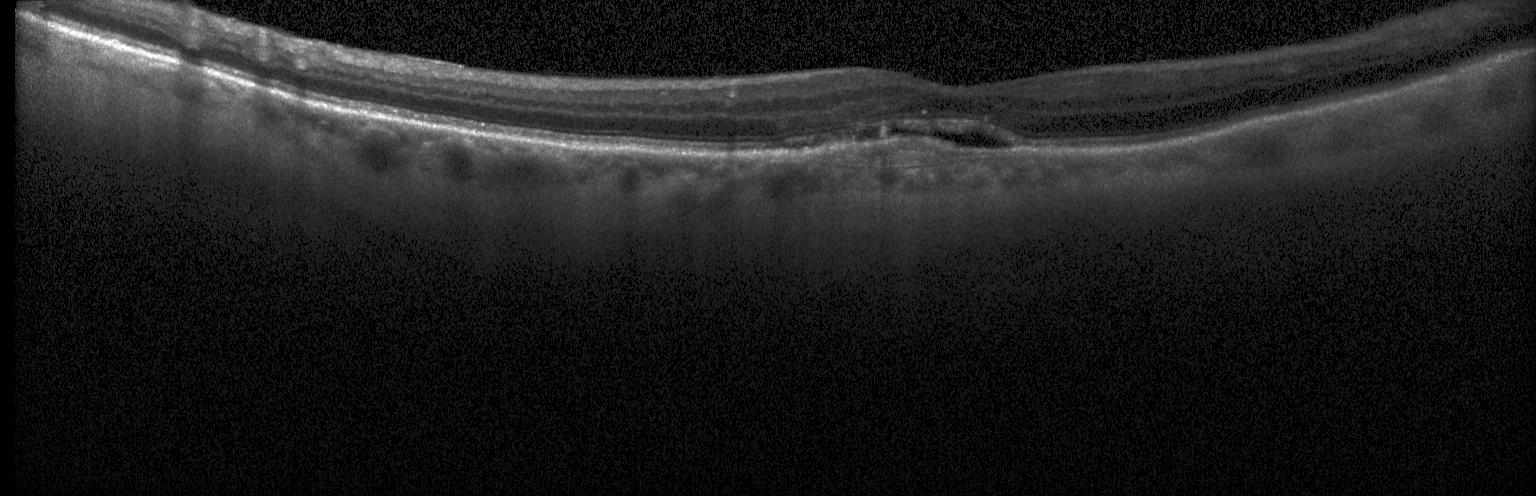

Retinal OCT cross-section showing choroidal neovascularization.